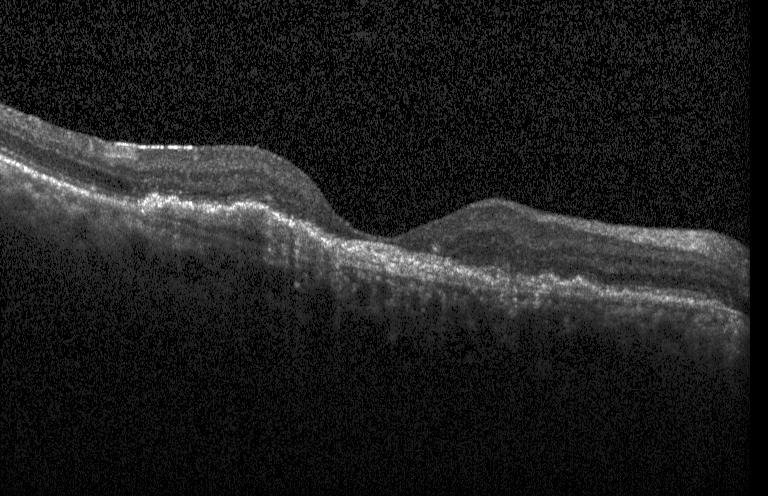
OCT line scan · Heidelberg Spectralis · macular scan.
Diagnosis: choroidal neovascularization.